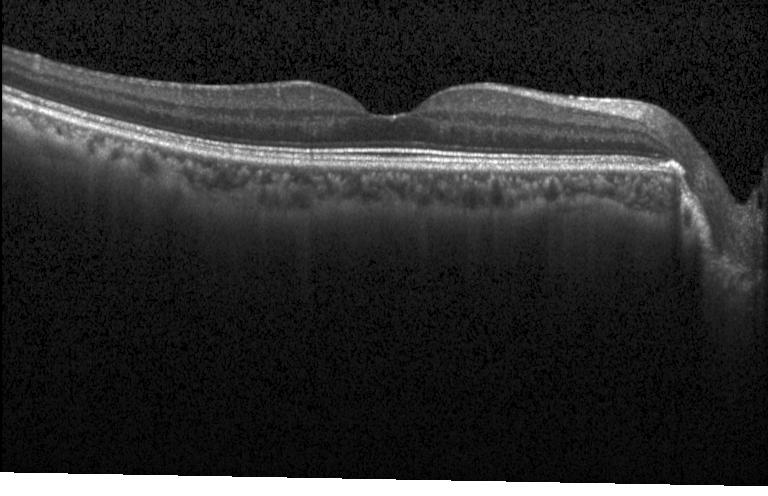

Impression: no evidence of choroidal neovascularization, diabetic macular edema, or drusen.